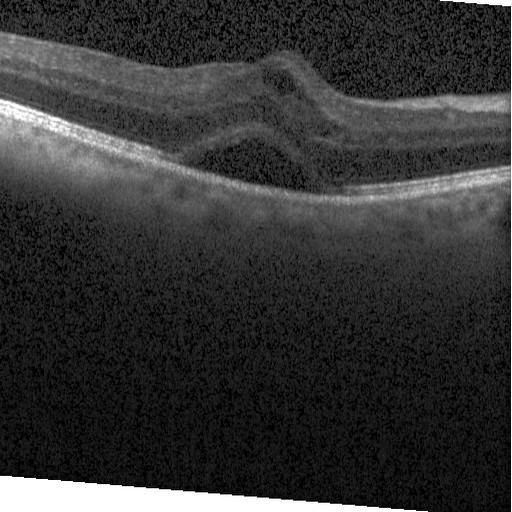 This B-scan demonstrates diabetic macular edema (DME).